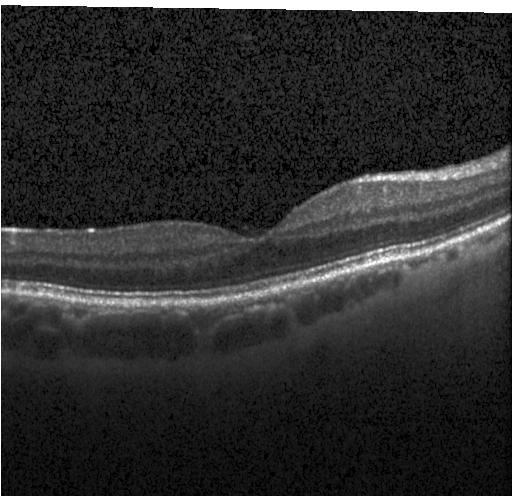

Macular scan. SD-OCT. OCT line scan
No CNV, no DME, and no drusen.